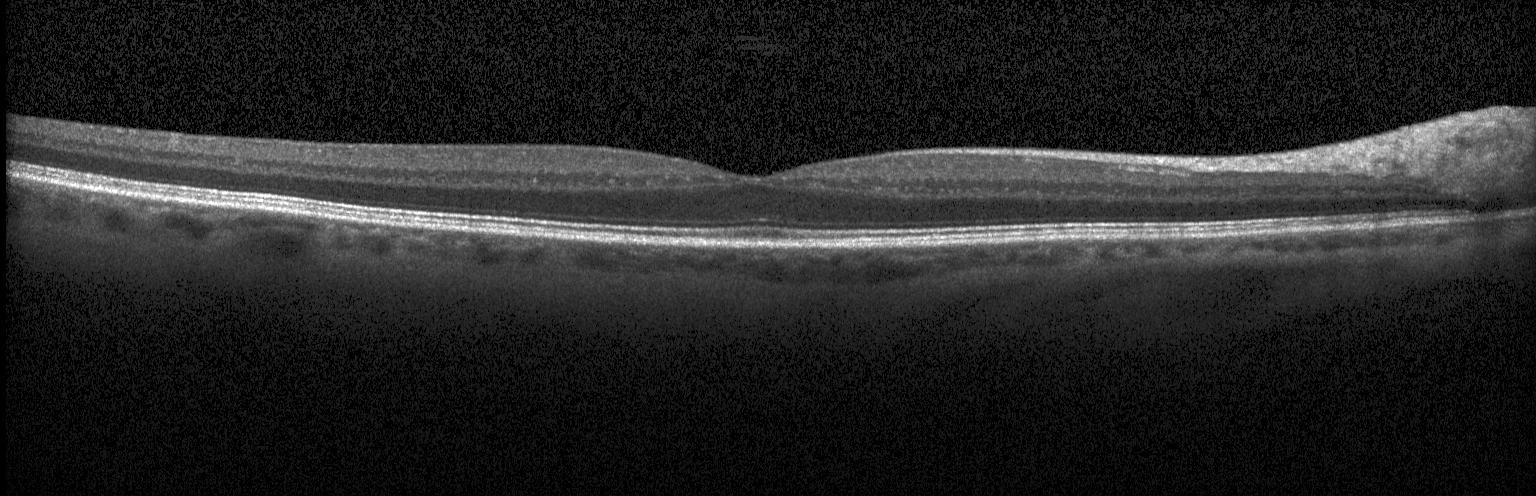

OCT finding: no choroidal neovascularization, no diabetic macular edema, and no drusen.